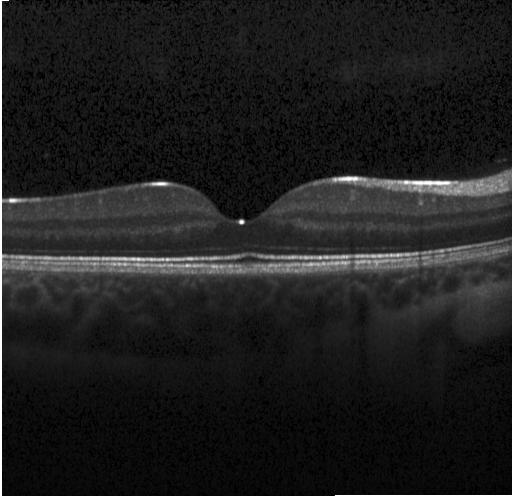
Impression: no evidence of CNV, DME, or drusen.